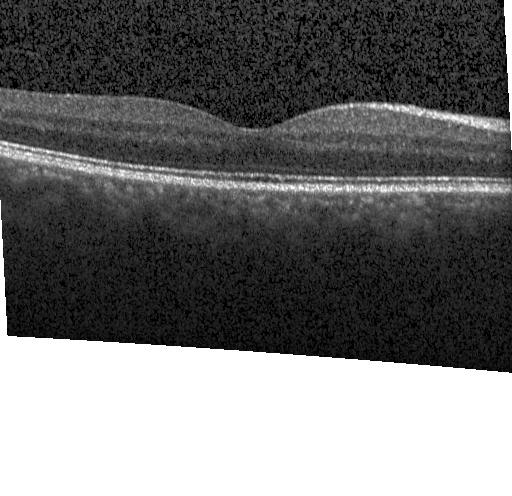
Optical coherence tomography scan, through the macula.
Assessment: neither CNV, DME, nor drusen.